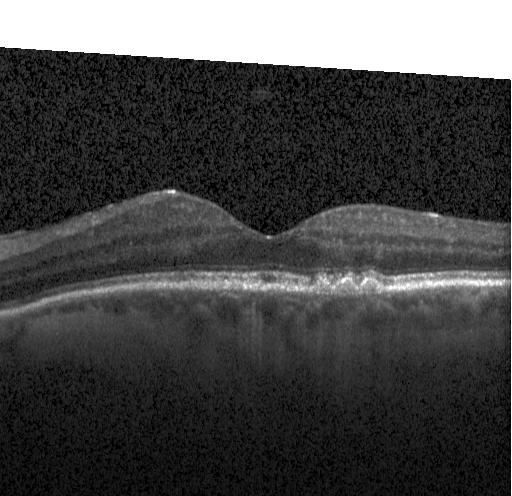

Spectral-domain OCT B-scan: sub-RPE drusenoid deposits.